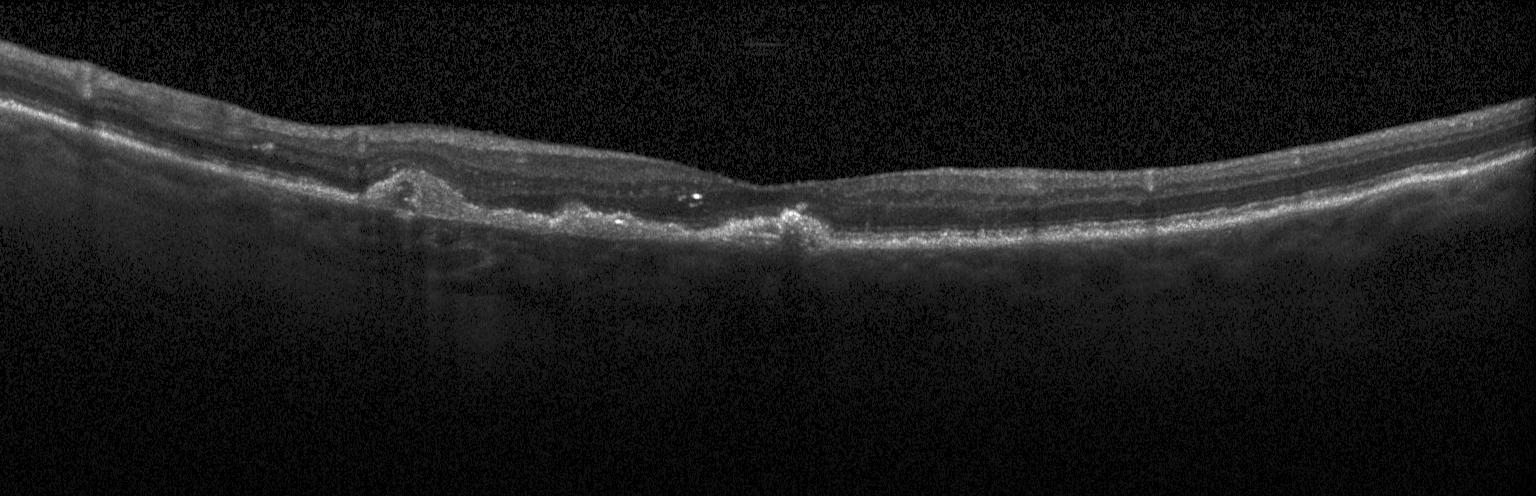 OCT line scan. Spectral-domain OCT. Acquired on a Heidelberg Spectralis. Through the macula. The scan shows choroidal neovascularization (CNV).